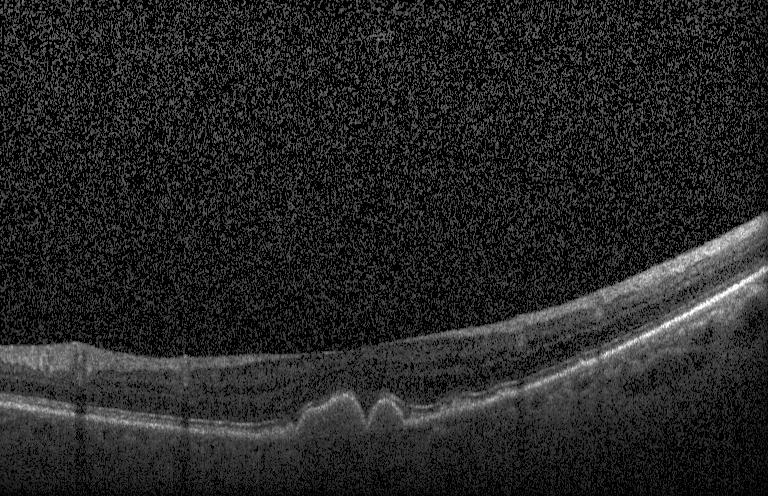 Retinal OCT cross-section.
Finding: sub-RPE drusenoid deposits.